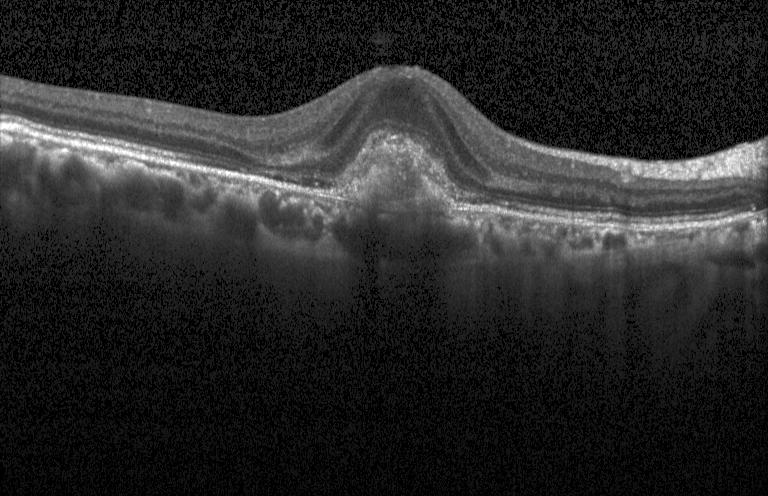

Spectral-domain optical coherence tomography, fovea-centered, OCT B-scan. OCT finding: CNV.